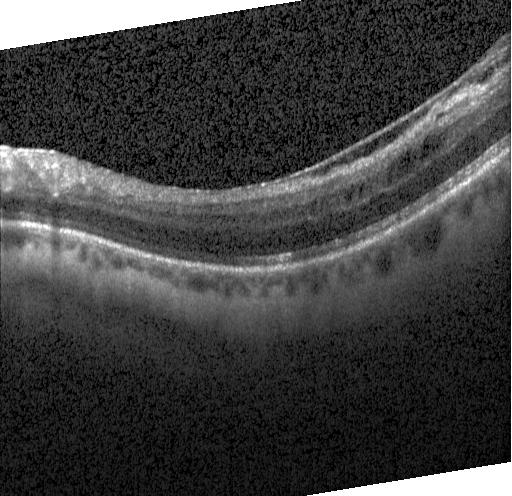
Macular OCT: diabetic macular edema (DME).